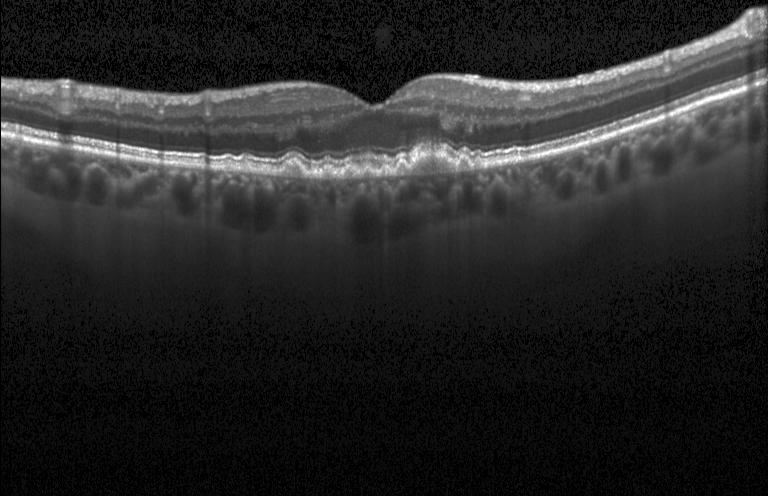

Macular OCT: sub-RPE drusenoid deposits.